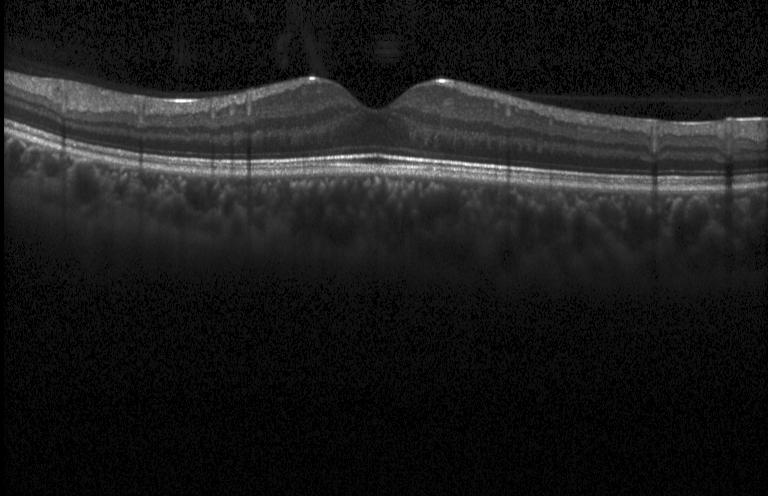 Optical coherence tomography B-scan.
Macular OCT: no CNV, no DME, and no drusen.